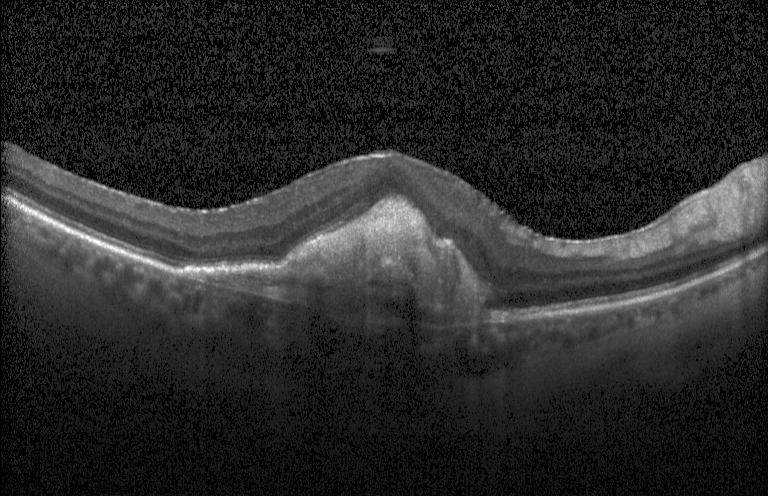
Spectral-domain OCT · retinal OCT cross-section
Finding: a choroidal neovascular membrane.